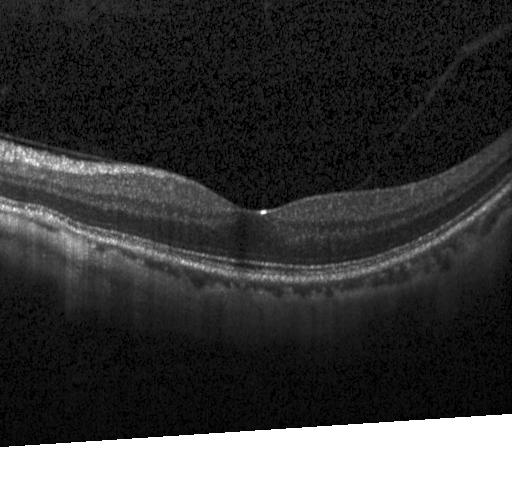

Macular OCT demonstrating no choroidal neovascularization, diabetic macular edema, or drusen.